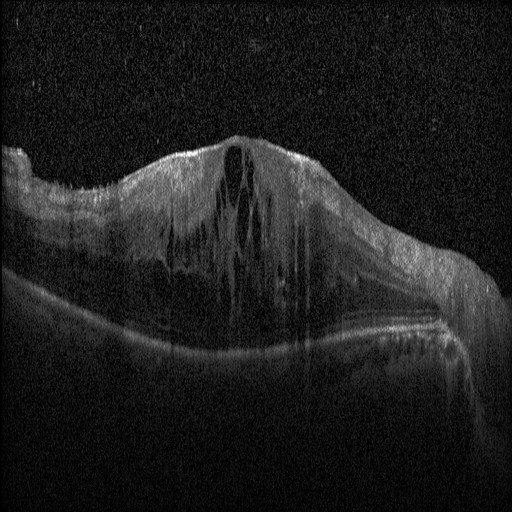 SD-OCT. Acquired on a Heidelberg Spectralis. Horizontal scan through the fovea. OCT line scan — Finding: diabetic macular edema (DME).